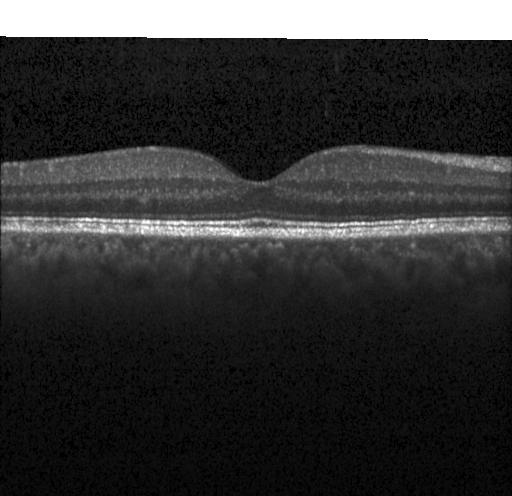
Impression: neither CNV, DME, nor drusen.